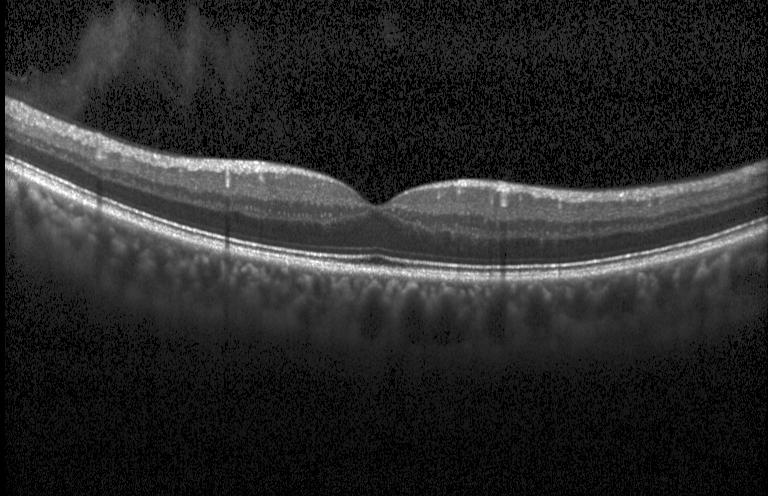
Through the macula; spectral-domain optical coherence tomography; Heidelberg Spectralis; optical coherence tomography scan — OCT finding: no evidence of CNV, DME, or drusen.